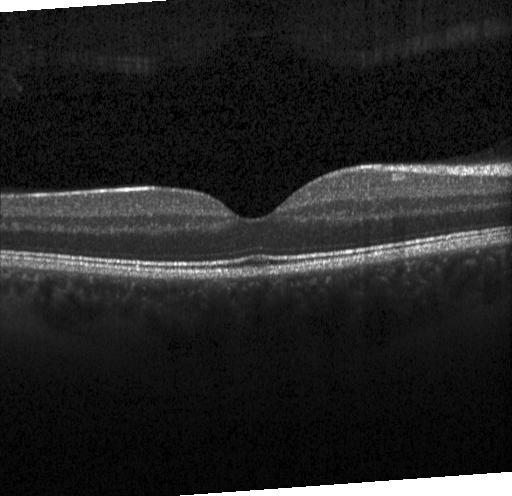

Optical coherence tomography B-scan — Macular OCT: neither choroidal neovascularization, diabetic macular edema, nor drusen.